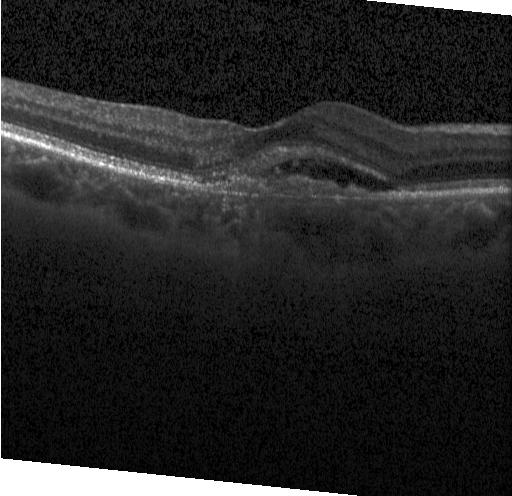

Impression: a choroidal neovascular membrane.